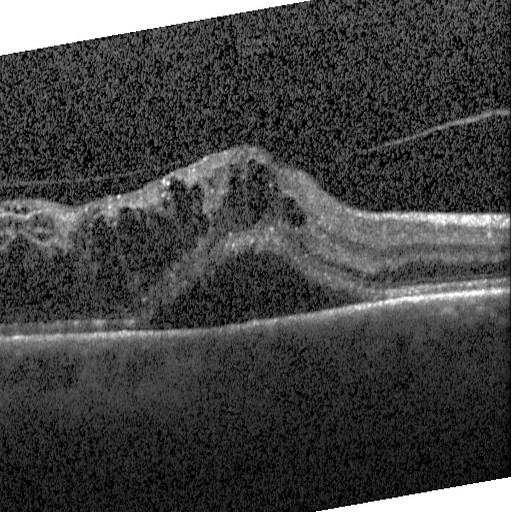
OCT line scan
The scan shows diabetic macular edema.